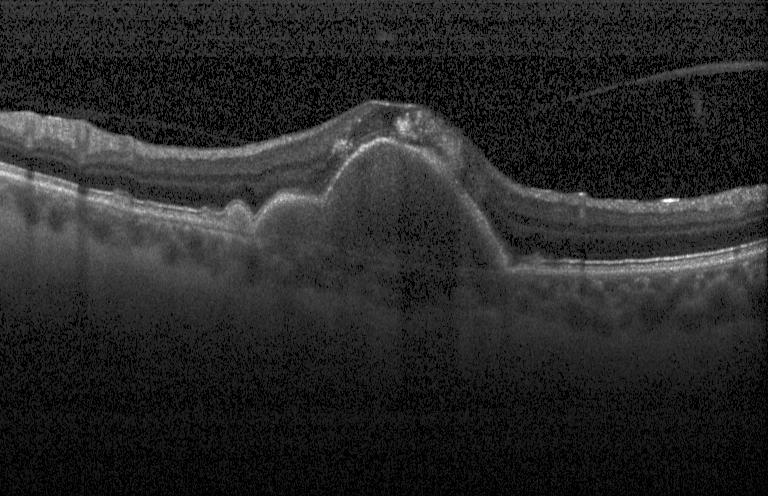 Dx: CNV.